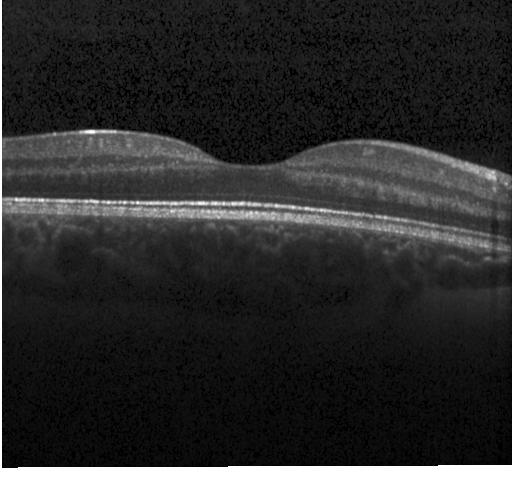 Macular scan. OCT B-scan.
No evidence of CNV, DME, or drusen.